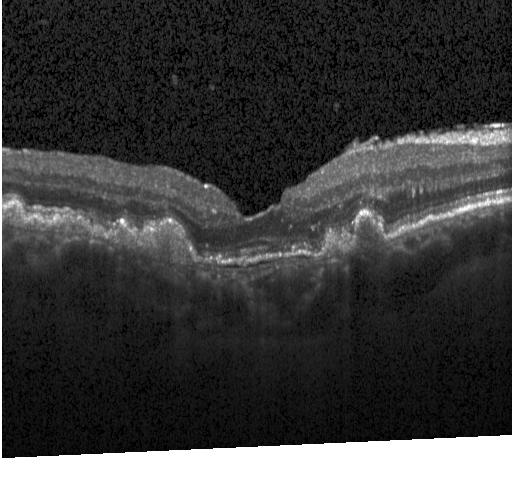 Macular OCT: choroidal neovascularization.